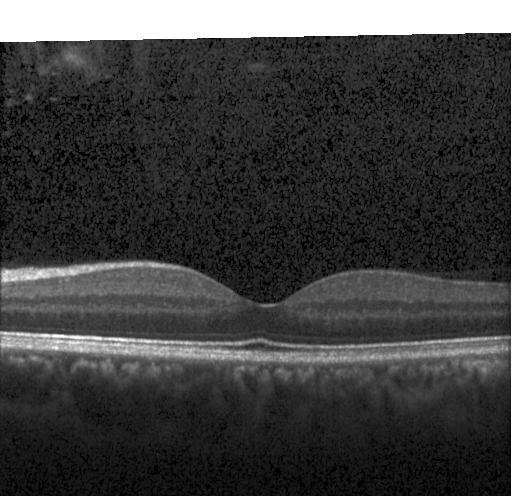 Retinal OCT B-scan — Diagnosis: no evidence of CNV, DME, or drusen.